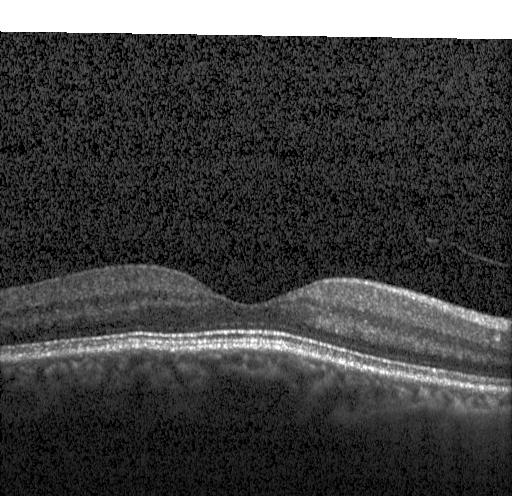

Spectral-domain OCT; OCT B-scan; acquired on a Heidelberg Spectralis; through the macula.
Diagnosis: no choroidal neovascularization, no diabetic macular edema, and no drusen.